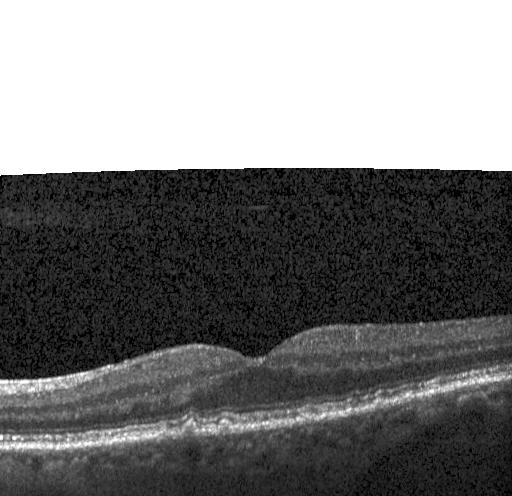
Centered on the fovea · instrument: Heidelberg Spectralis · retinal OCT B-scan · spectral-domain OCT.
Finding: drusen.